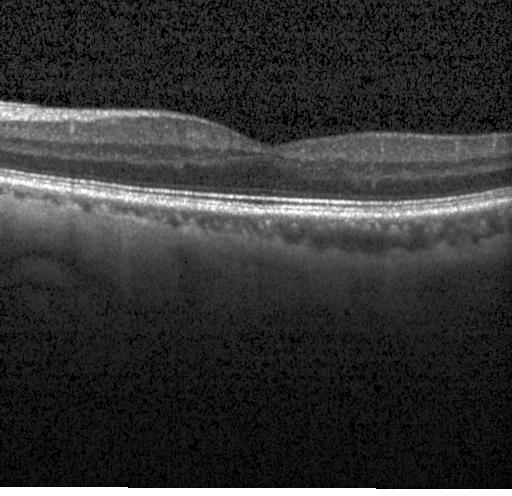 Spectral-domain OCT B-scan: no choroidal neovascularization, no diabetic macular edema, and no drusen.